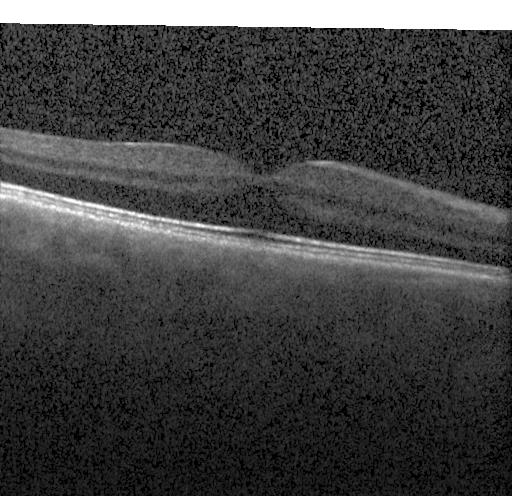

OCT B-scan
This B-scan demonstrates no evidence of choroidal neovascularization, diabetic macular edema, or drusen.